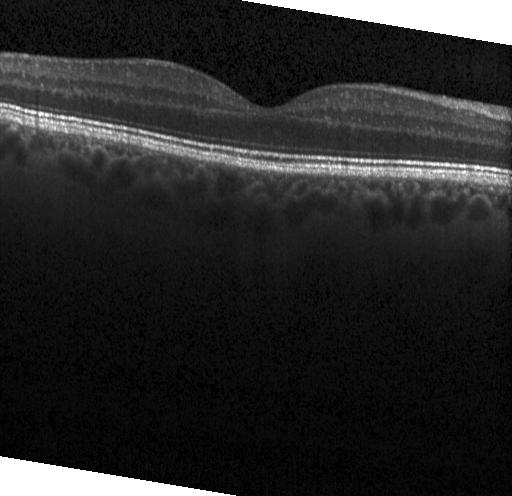

SD-OCT. Retinal OCT B-scan.
Impression: no CNV, no DME, and no drusen.